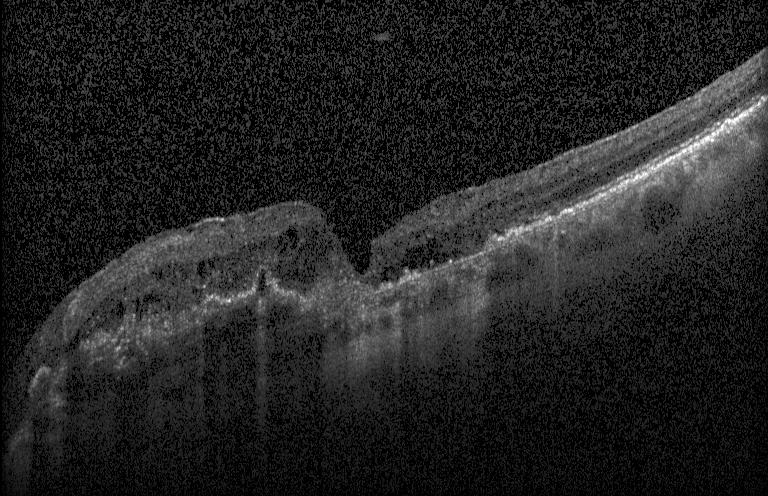 Acquired on a Heidelberg Spectralis. Macular scan. Optical coherence tomography B-scan. Spectral-domain OCT — The scan shows a choroidal neovascular membrane.